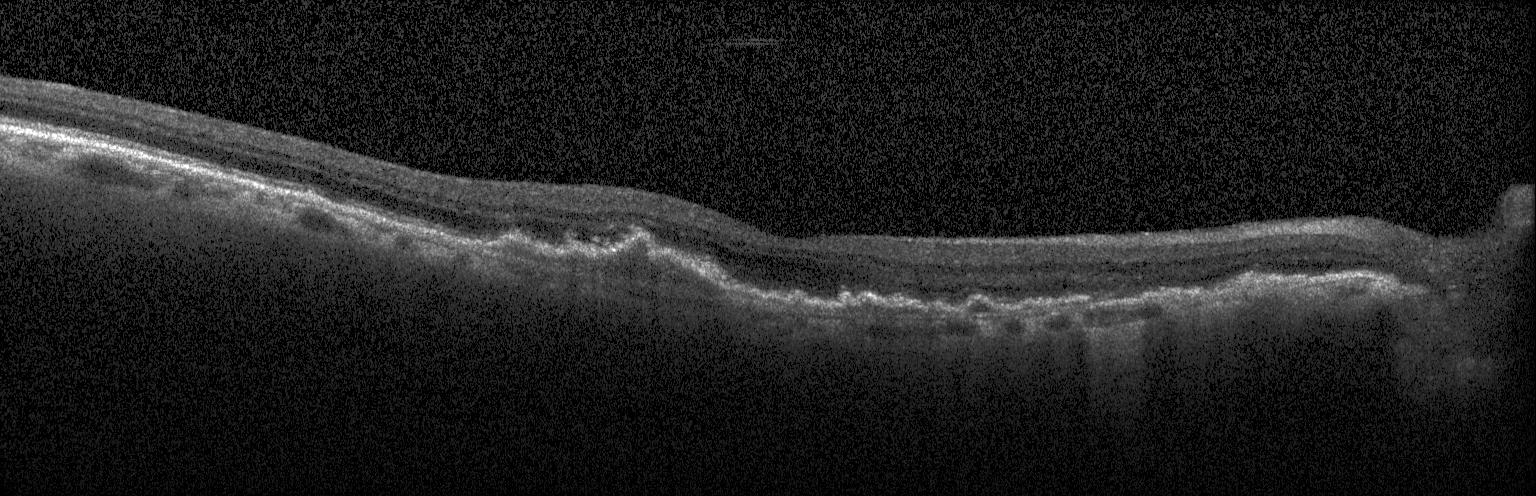
Centered on the fovea, retinal OCT cross-section, Heidelberg Spectralis OCT system
Finding: choroidal neovascularization (CNV).